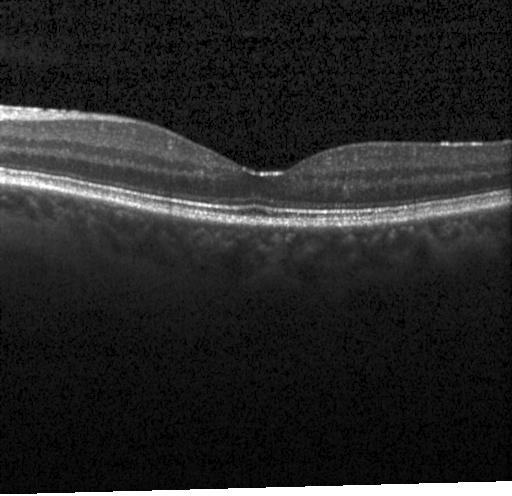

Impression: no choroidal neovascularization, diabetic macular edema, or drusen.